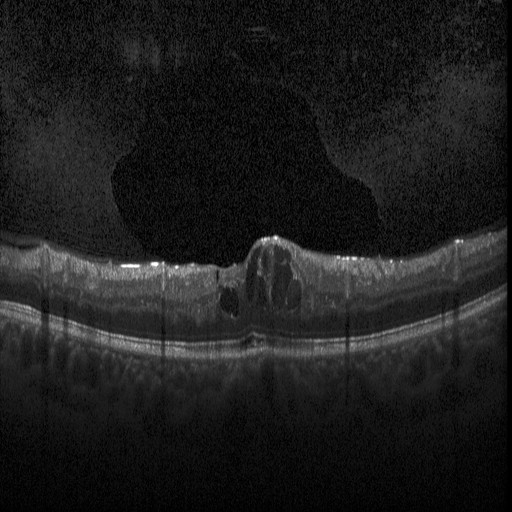
Optical coherence tomography B-scan. Diabetic macular edema (DME).